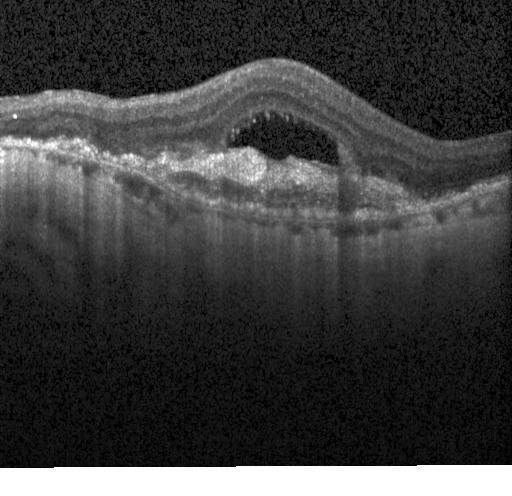
Diagnosis: a choroidal neovascular membrane.